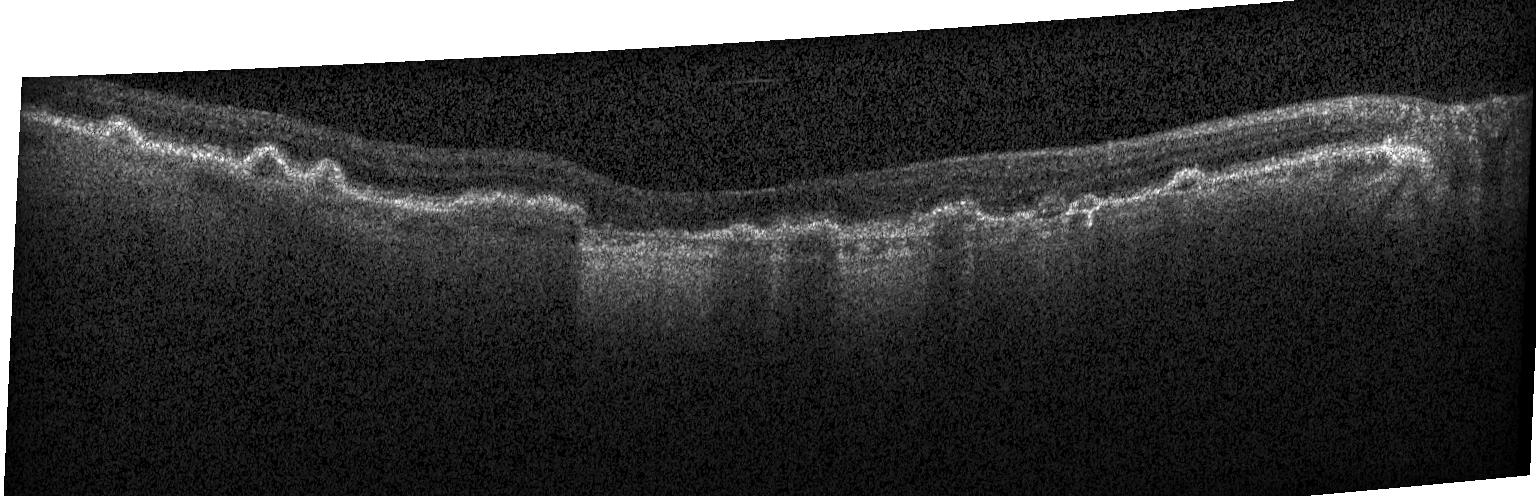
Macular scan · retinal OCT B-scan. Dx: choroidal neovascularization (CNV).